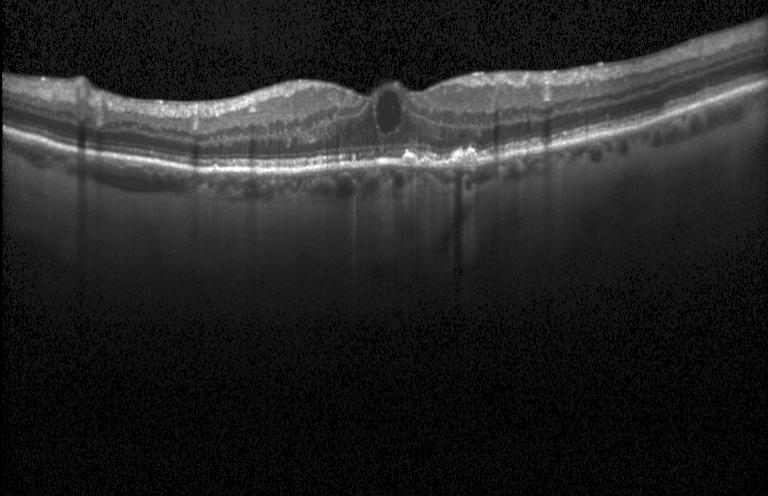

Macular scan · optical coherence tomography scan · Heidelberg Spectralis — Diagnosis: a choroidal neovascular membrane.